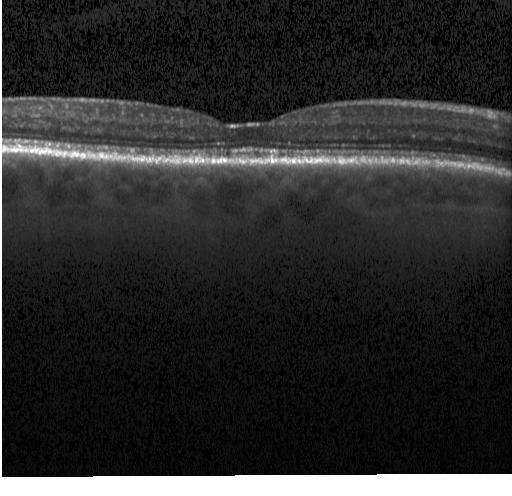
Optical coherence tomography scan; macular scan; spectral-domain OCT
Dx: no evidence of CNV, DME, or drusen.